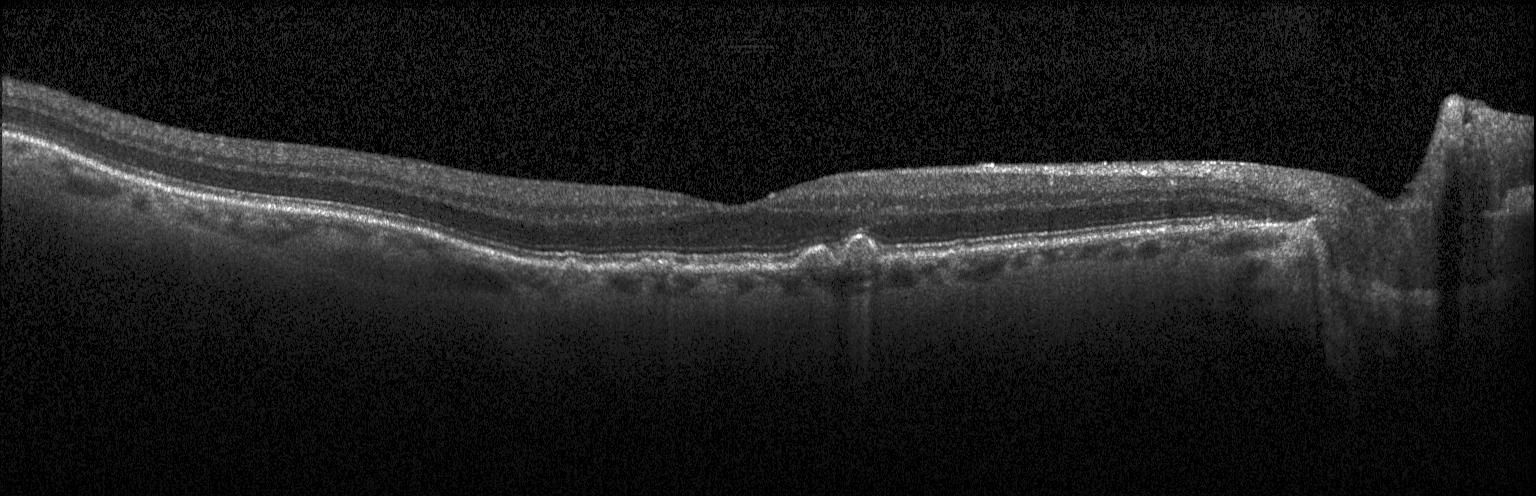

Spectral-domain OCT B-scan: sub-RPE drusenoid deposits.